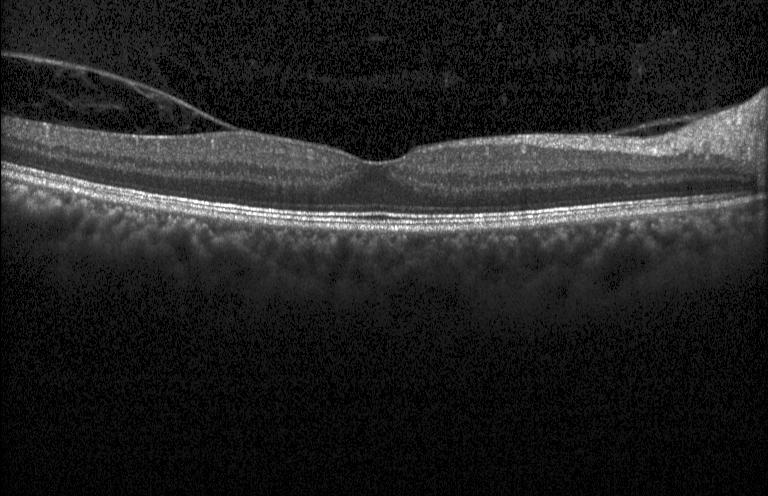
OCT line scan.
Diagnosis: no choroidal neovascularization, diabetic macular edema, or drusen.